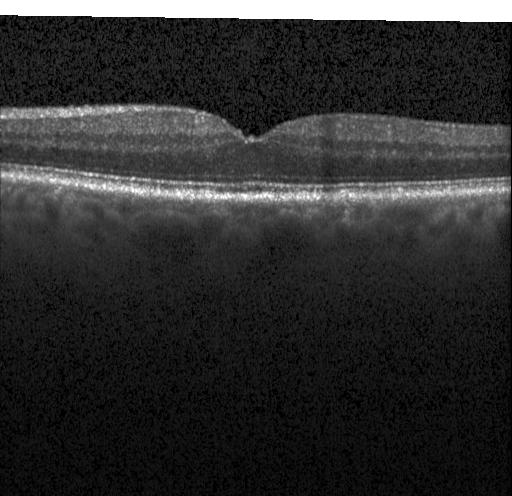

No choroidal neovascularization, diabetic macular edema, or drusen.